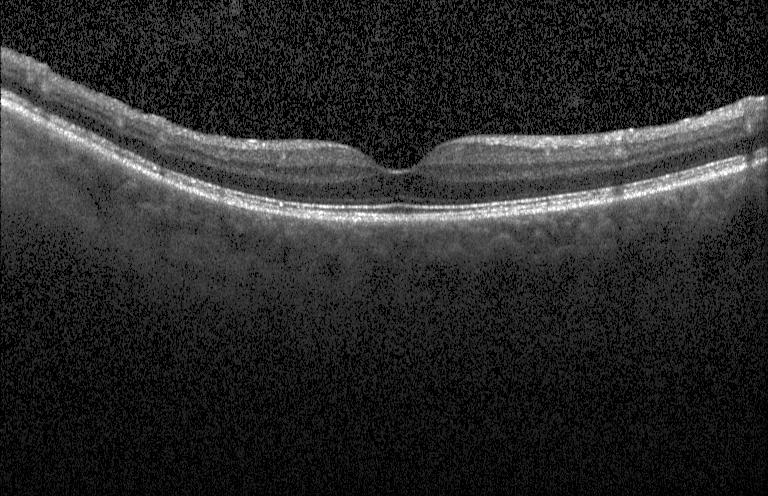
Through the macula; optical coherence tomography scan.
Finding: no evidence of choroidal neovascularization, diabetic macular edema, or drusen.